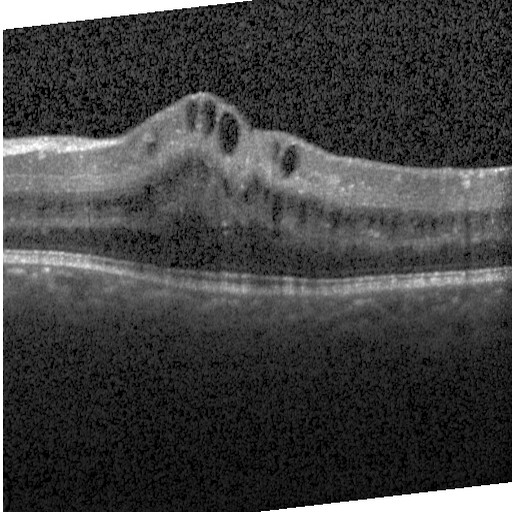

Retinal OCT cross-section. DME.